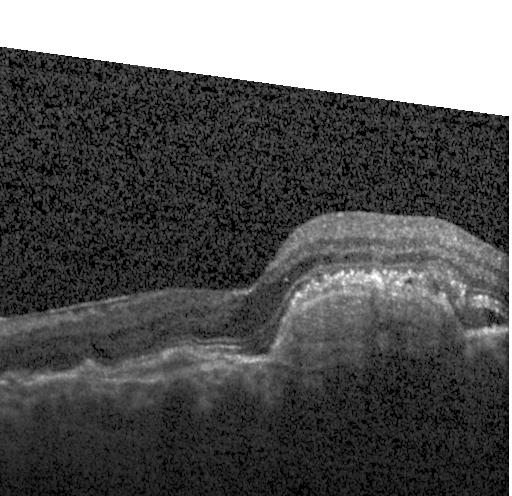 Optical coherence tomography B-scan
Impression: choroidal neovascularization.